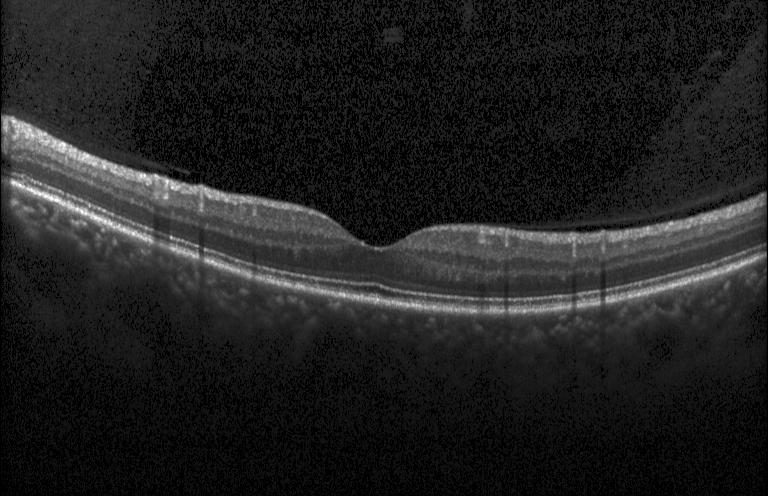
Macular scan, Heidelberg Spectralis, OCT line scan, spectral-domain optical coherence tomography.
Assessment: neither choroidal neovascularization, diabetic macular edema, nor drusen.